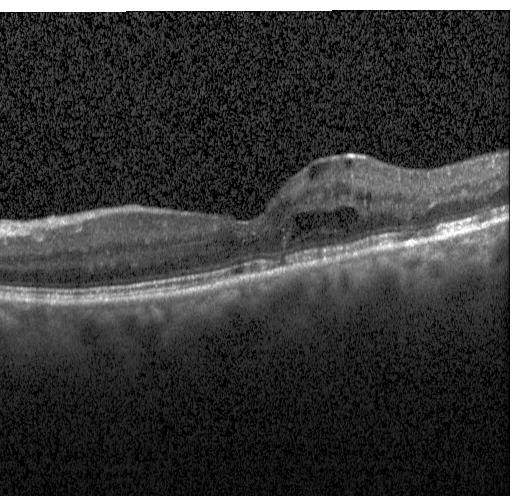
Optical coherence tomography B-scan.
Finding: DME.